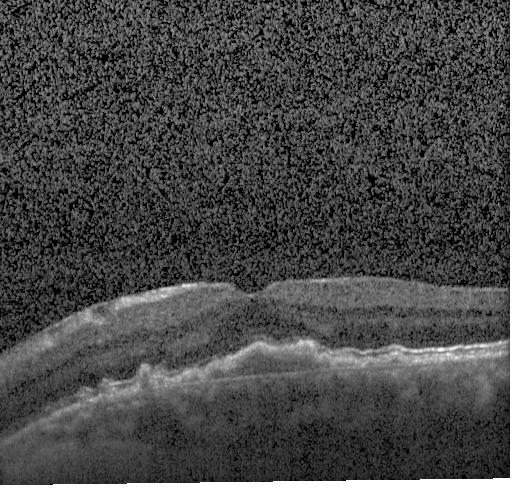 This B-scan demonstrates a choroidal neovascular membrane.